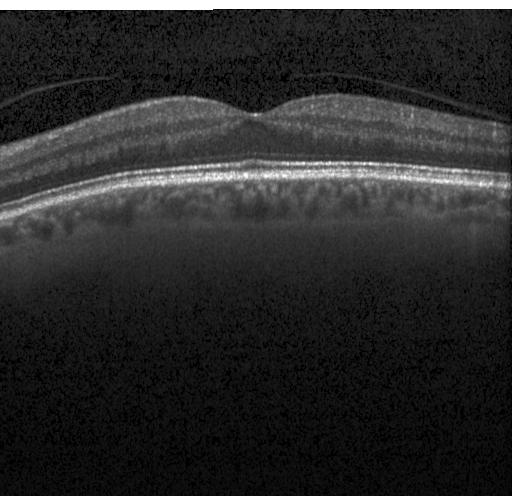
Retinal OCT cross-section showing neither CNV, DME, nor drusen.